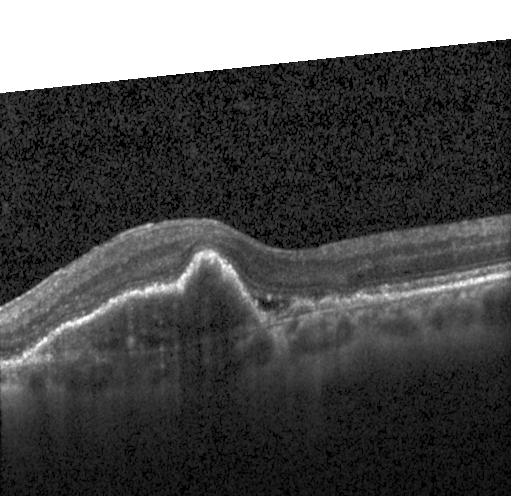 Macular OCT: a choroidal neovascular membrane.